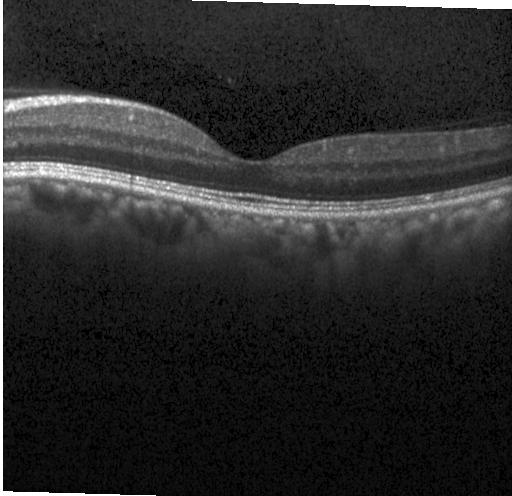 Retinal OCT cross-section. Dx: no choroidal neovascularization, no diabetic macular edema, and no drusen.